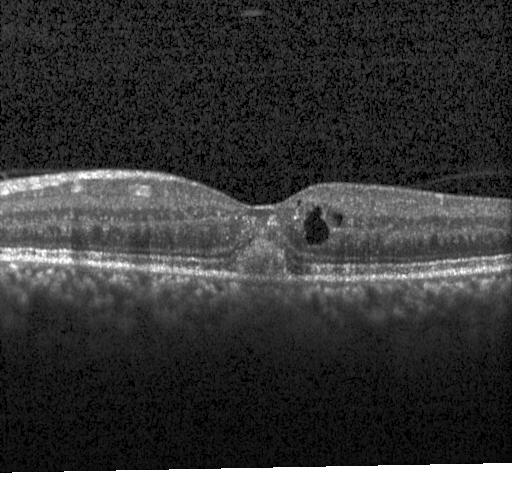
Assessment: a choroidal neovascular membrane.